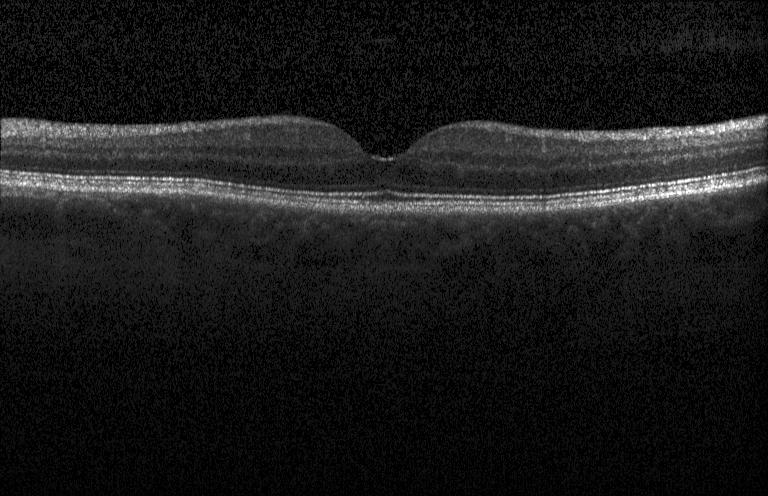 Macular OCT: no choroidal neovascularization, no diabetic macular edema, and no drusen.